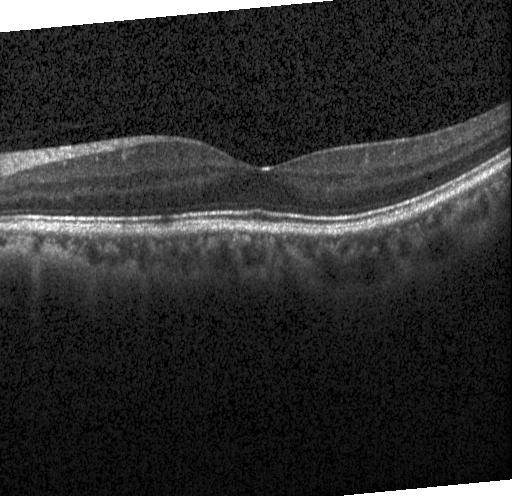

Macular OCT: no evidence of choroidal neovascularization, diabetic macular edema, or drusen.